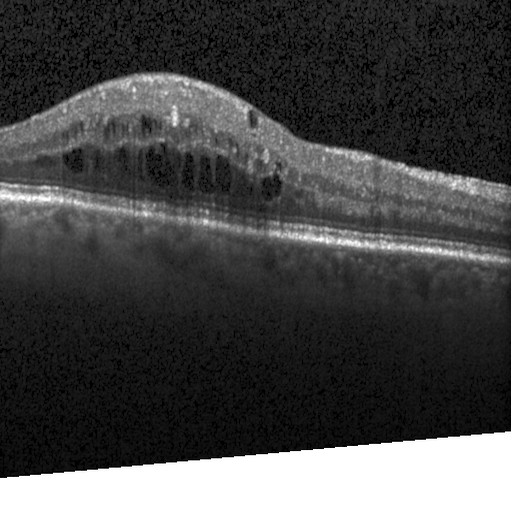 OCT scan showing diabetic macular edema.